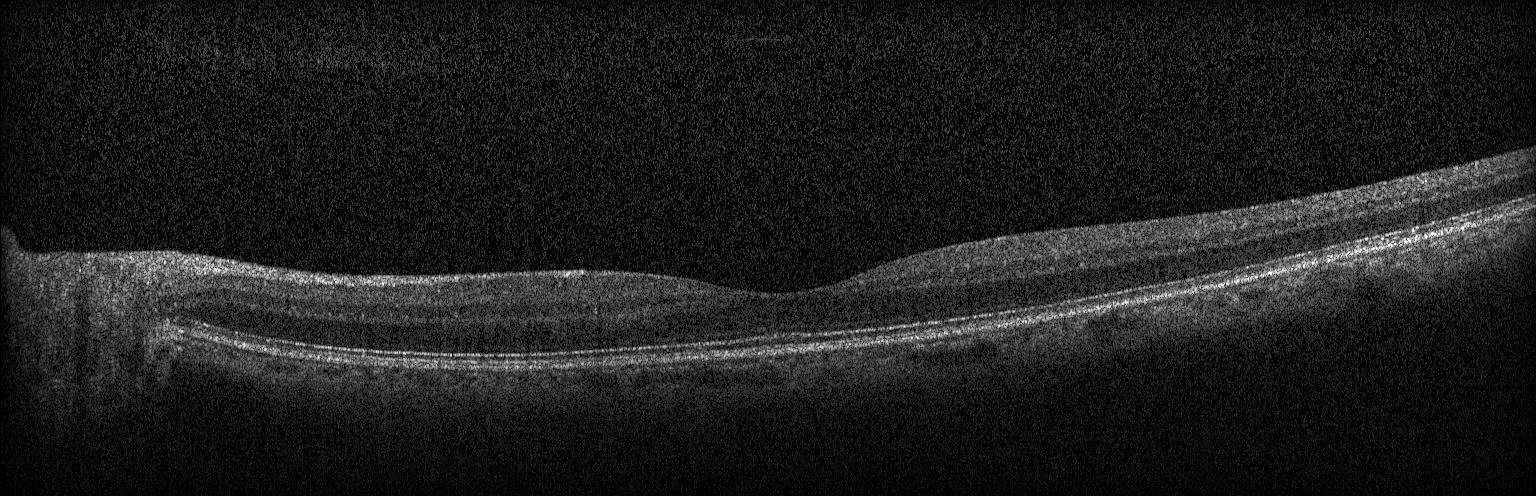

Optical coherence tomography scan; SD-OCT; instrument: Heidelberg Spectralis; horizontal scan through the fovea
Assessment: neither choroidal neovascularization, diabetic macular edema, nor drusen.